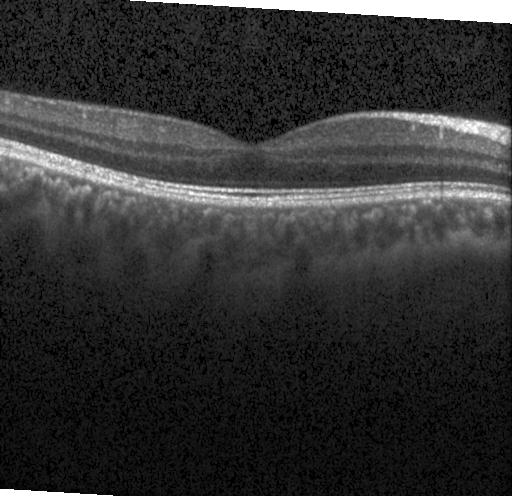 Macular scan; OCT line scan.
Impression: neither choroidal neovascularization, diabetic macular edema, nor drusen.